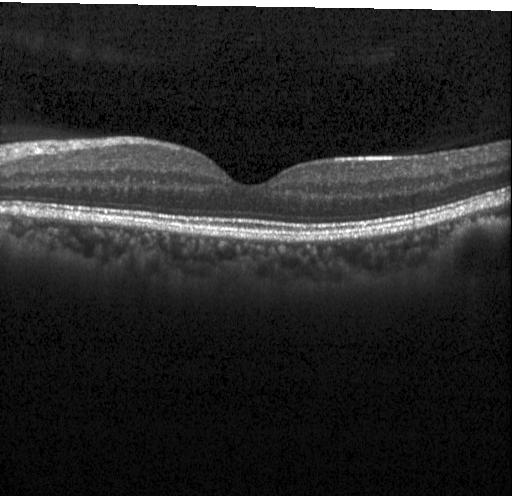 Acquired on a Heidelberg Spectralis. Horizontal scan through the fovea. Spectral-domain optical coherence tomography. Retinal OCT B-scan.
Finding: no choroidal neovascularization, no diabetic macular edema, and no drusen.